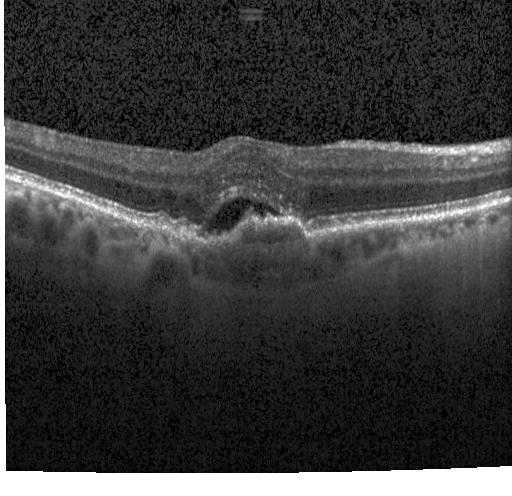
Acquired on a Heidelberg Spectralis. Horizontal scan through the fovea. OCT B-scan. SD-OCT
Impression: a choroidal neovascular membrane.